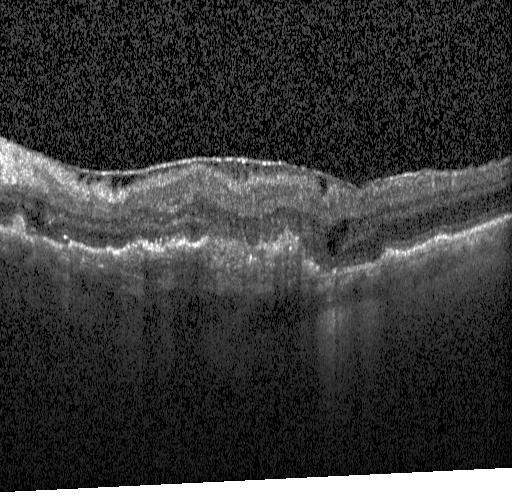
Optical coherence tomography scan.
Impression: a choroidal neovascular membrane.